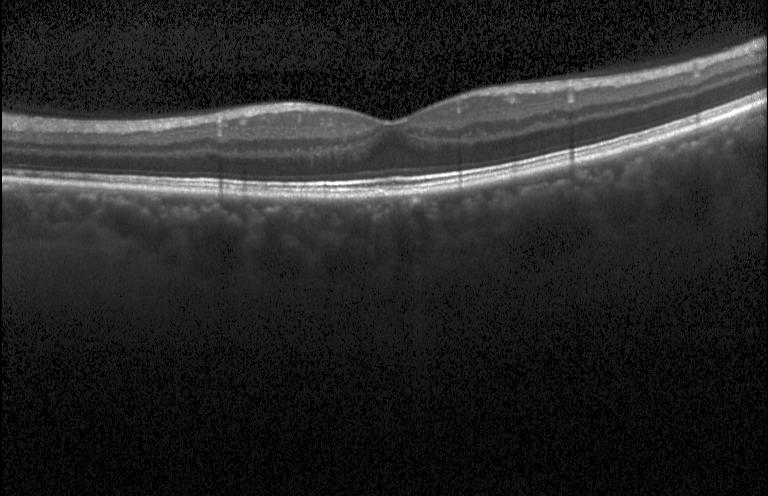 Heidelberg Spectralis; OCT line scan; macular scan.
Impression: no evidence of choroidal neovascularization, diabetic macular edema, or drusen.